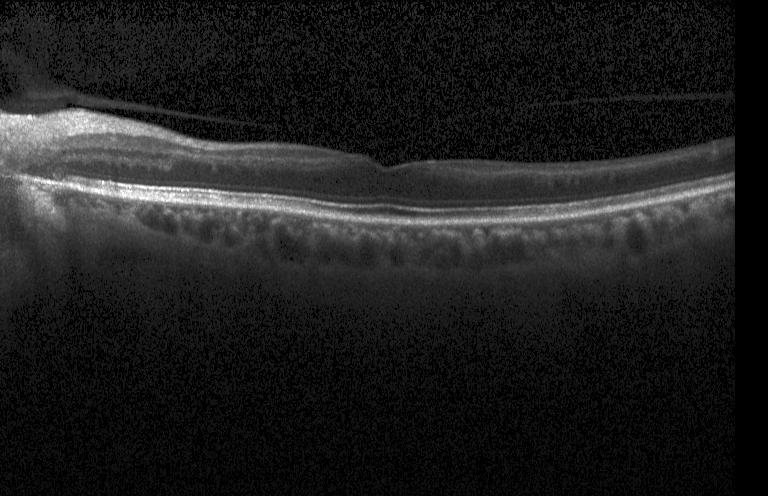 Finding: no choroidal neovascularization, no diabetic macular edema, and no drusen.